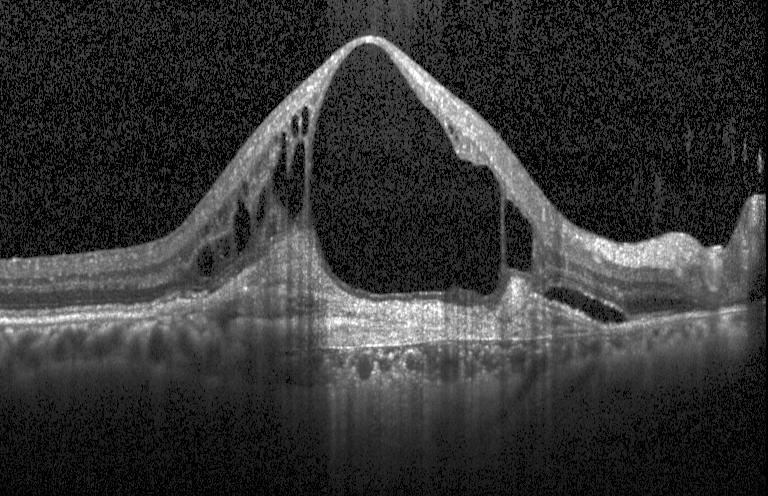

Instrument: Heidelberg Spectralis, retinal OCT cross-section
Diagnosis: choroidal neovascularization.